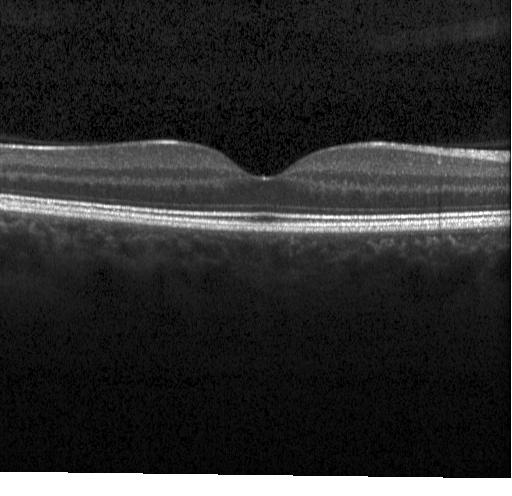

OCT B-scan
Assessment: neither CNV, DME, nor drusen.